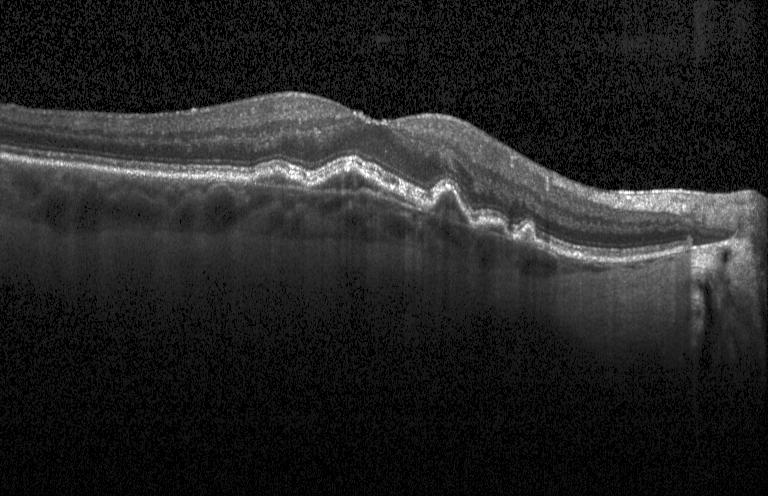
Dx: choroidal neovascularization (CNV).